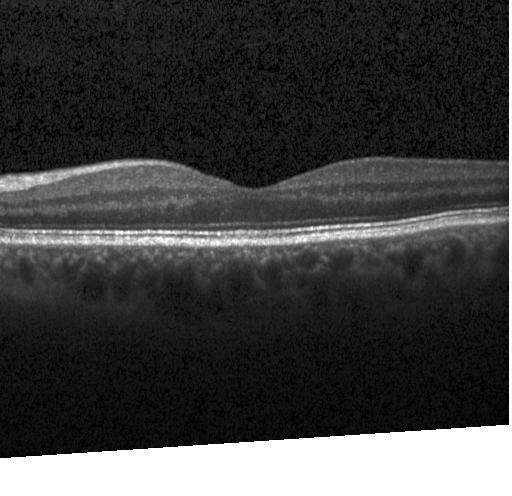 Optical coherence tomography scan; acquired on a Heidelberg Spectralis
No evidence of CNV, DME, or drusen.